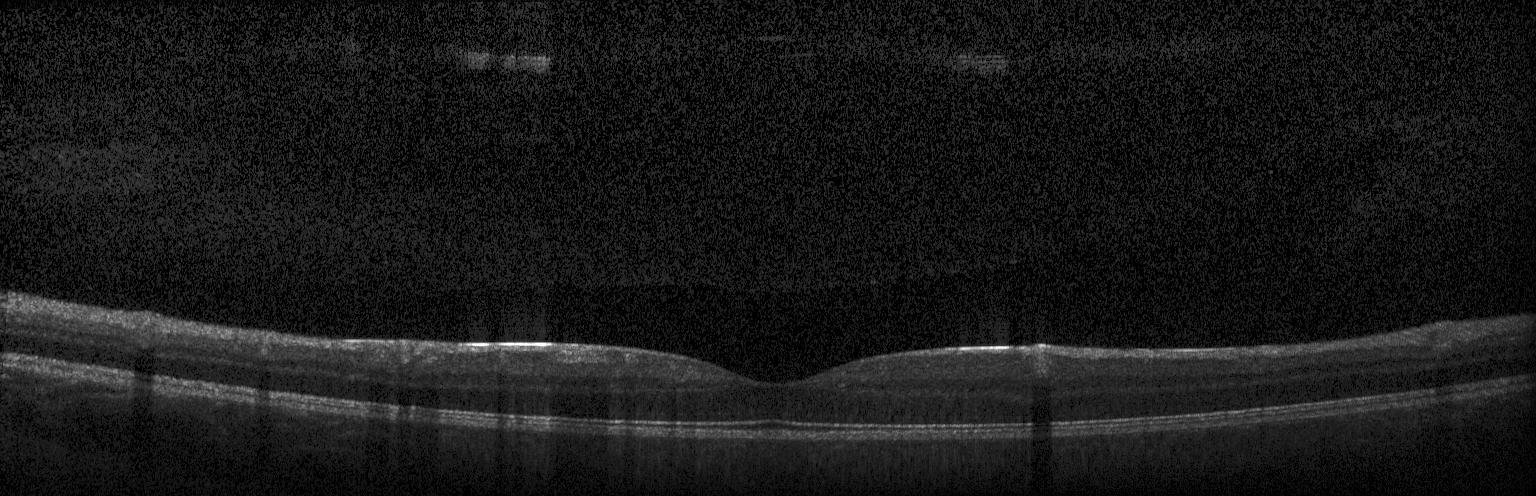 OCT finding: no choroidal neovascularization, diabetic macular edema, or drusen.